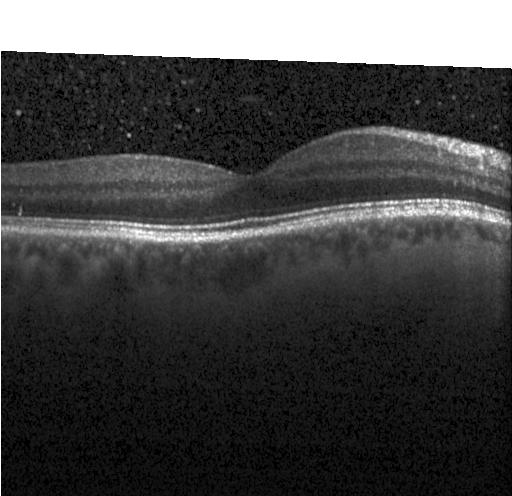

Spectral-domain optical coherence tomography; Heidelberg Spectralis OCT system; optical coherence tomography scan; horizontal scan through the fovea — Impression: no choroidal neovascularization, no diabetic macular edema, and no drusen.